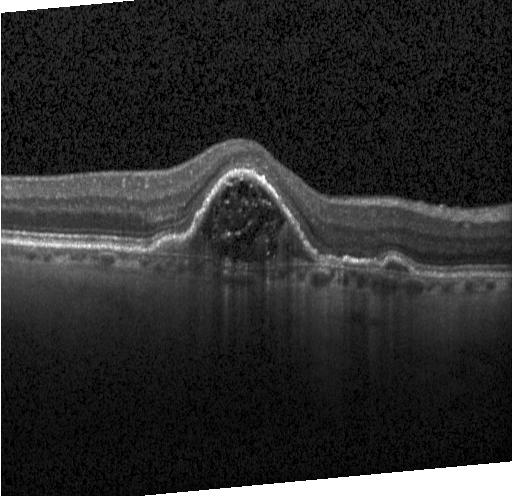

Optical coherence tomography scan. Choroidal neovascularization (CNV).